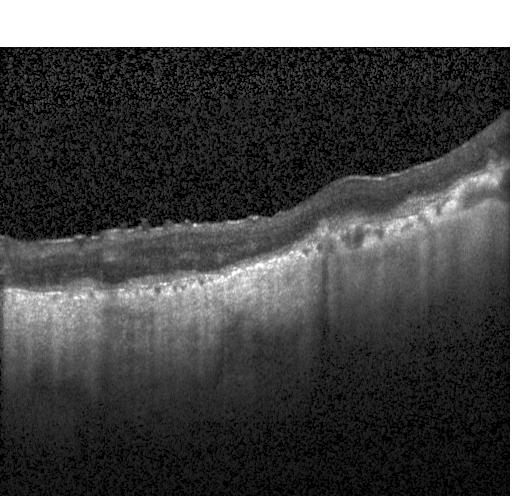 OCT line scan. Fovea-centered — Assessment: a choroidal neovascular membrane.